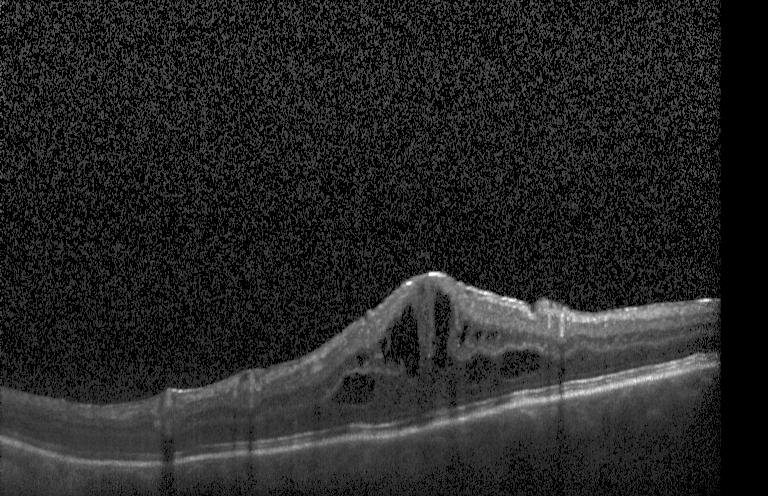
Retinal OCT B-scan. Centered on the fovea. Diagnosis: diabetic macular edema.